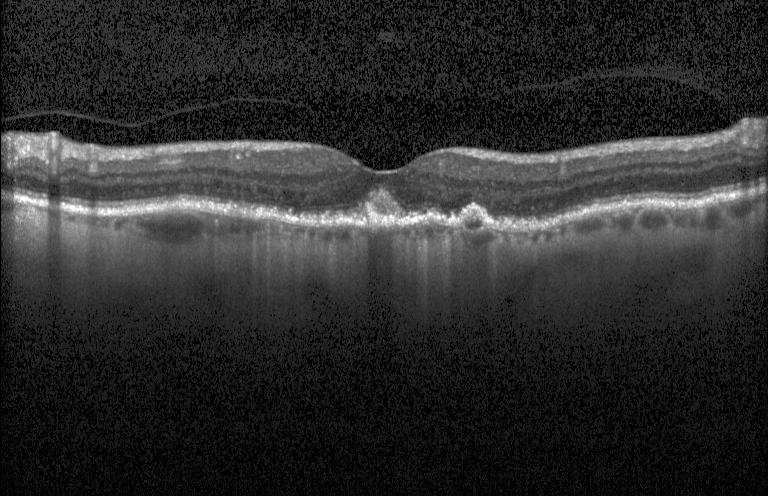
The scan shows multiple drusen.